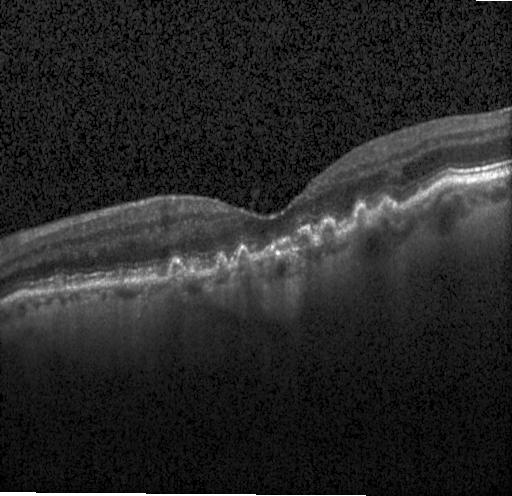 Fovea-centered, optical coherence tomography scan, spectral-domain OCT
Finding: drusen.